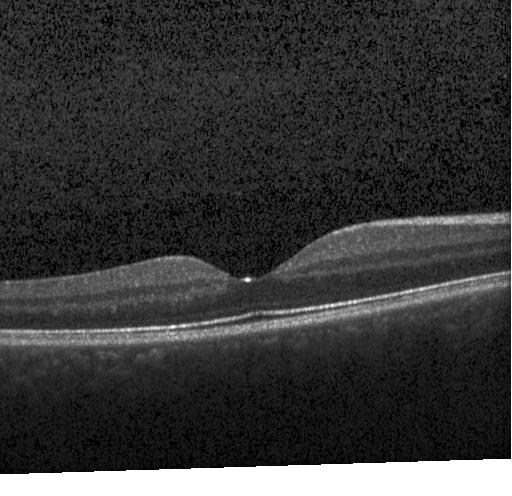
Optical coherence tomography B-scan
Impression: no choroidal neovascularization, no diabetic macular edema, and no drusen.